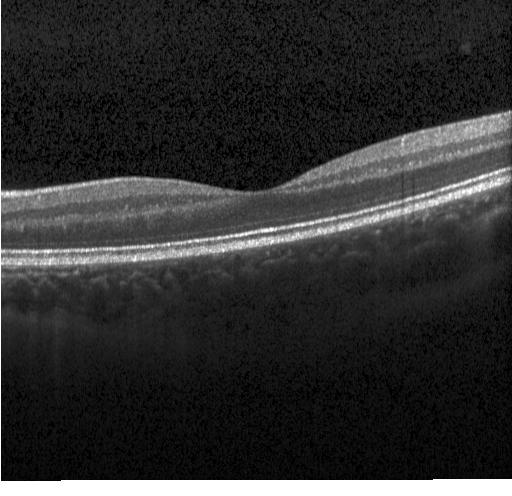

Impression: no evidence of choroidal neovascularization, diabetic macular edema, or drusen.